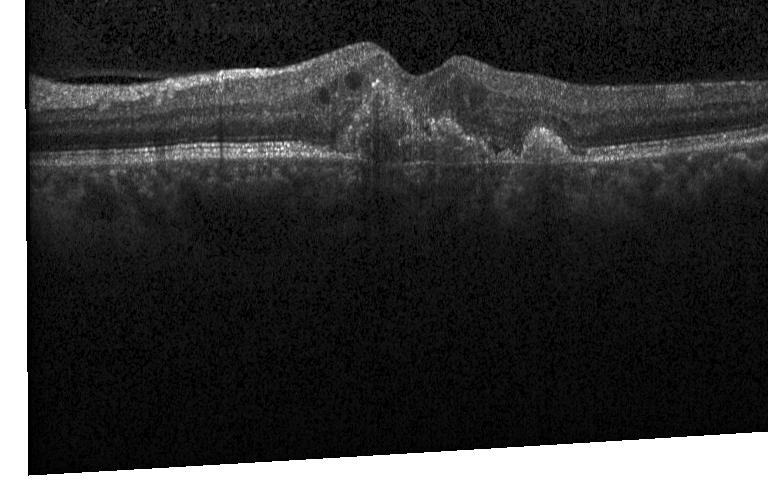

Spectral-domain OCT. Through the macula. Instrument: Heidelberg Spectralis. OCT B-scan. Dx: choroidal neovascularization (CNV).